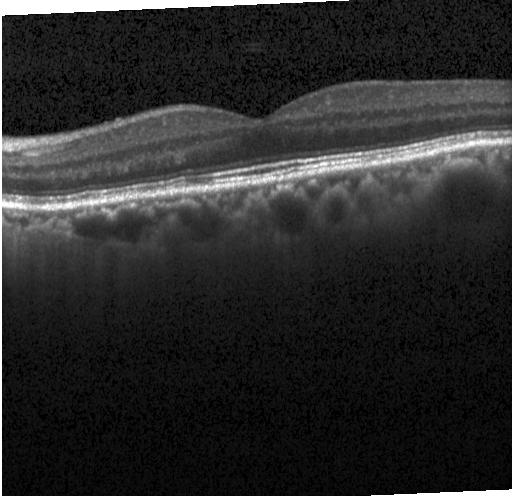 Spectral-domain OCT · instrument: Heidelberg Spectralis · OCT B-scan · through the macula.
Finding: no evidence of choroidal neovascularization, diabetic macular edema, or drusen.